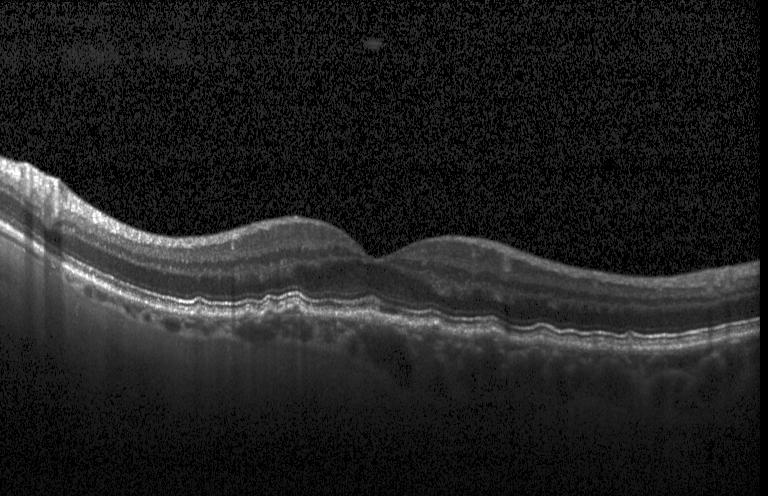
Drusen.